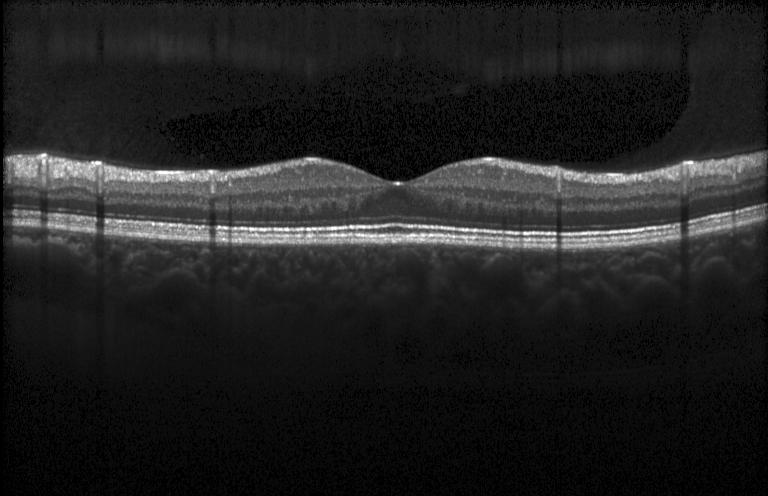 Spectral-domain OCT · OCT line scan. Finding: no choroidal neovascularization, no diabetic macular edema, and no drusen.